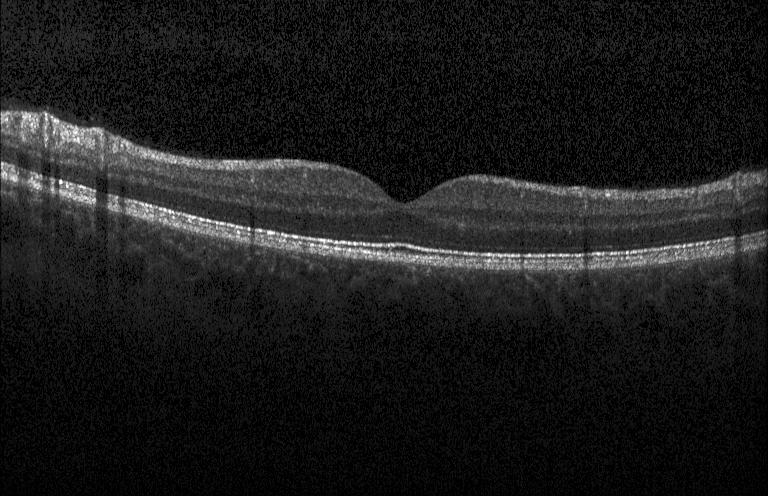
Spectral-domain optical coherence tomography. Retinal OCT cross-section. Macular scan — This B-scan demonstrates no CNV, DME, or drusen.